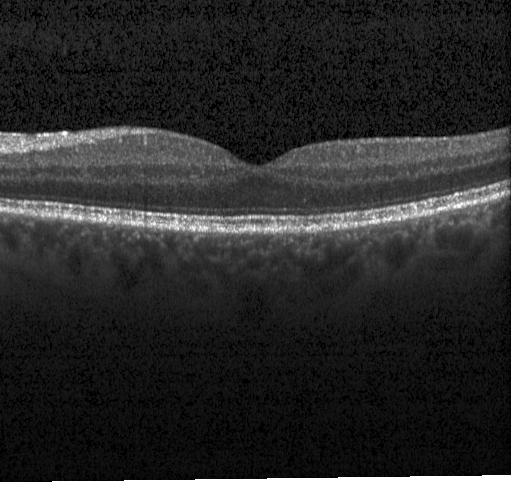
Impression: no evidence of choroidal neovascularization, diabetic macular edema, or drusen.